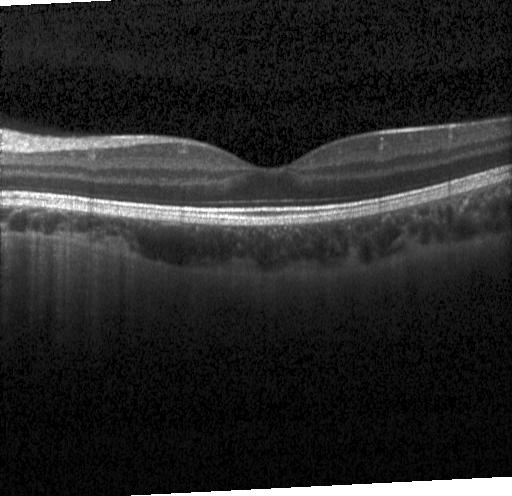 Spectral-domain OCT B-scan: neither CNV, DME, nor drusen.